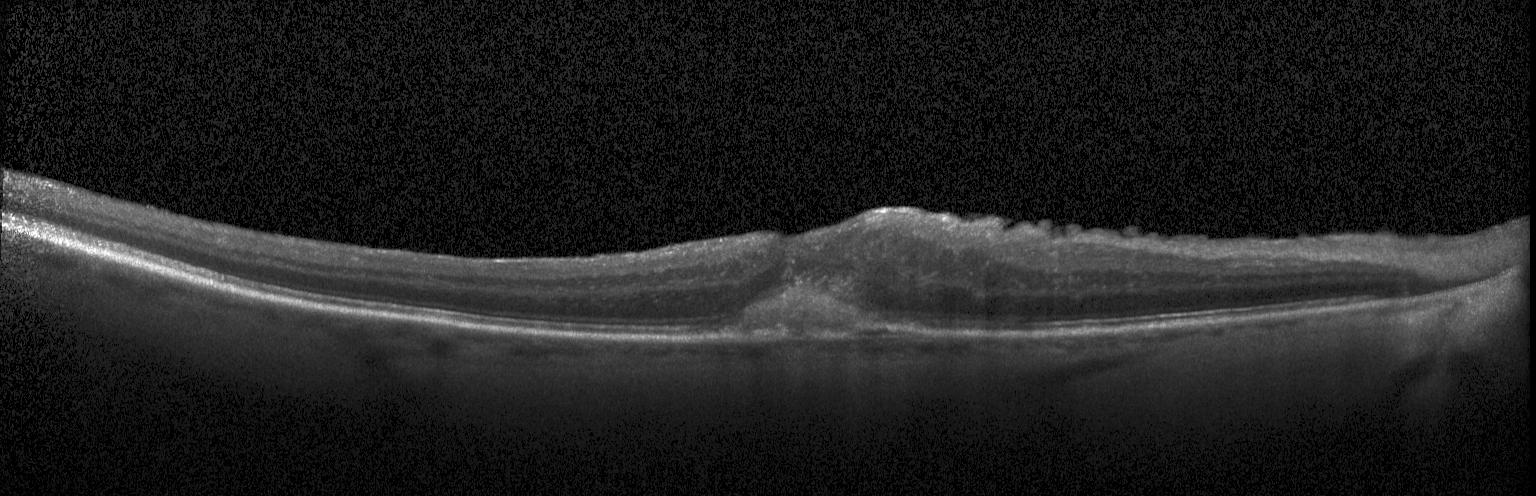
Spectral-domain optical coherence tomography, optical coherence tomography B-scan — The scan shows choroidal neovascularization (CNV).